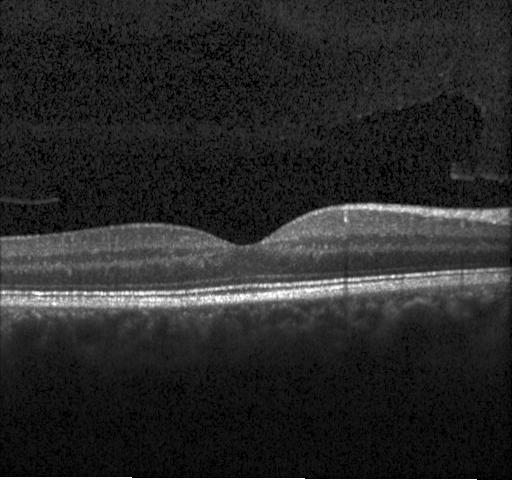 Fovea-centered; optical coherence tomography B-scan
Assessment: no choroidal neovascularization, diabetic macular edema, or drusen.